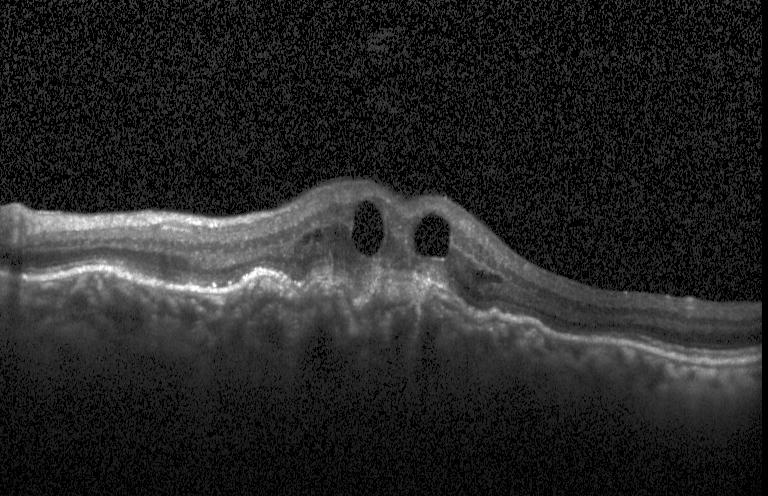 Finding: a choroidal neovascular membrane.